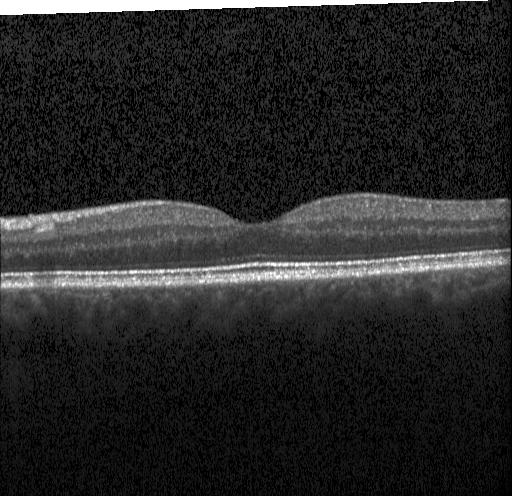 Optical coherence tomography B-scan — Impression: no choroidal neovascularization, no diabetic macular edema, and no drusen.